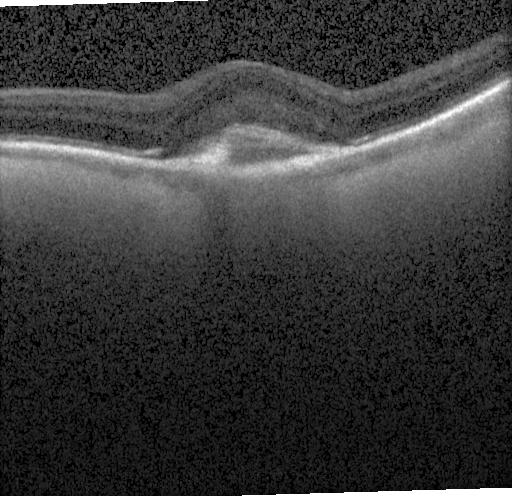 SD-OCT, horizontal scan through the fovea, retinal OCT B-scan, Heidelberg Spectralis OCT system — The scan shows a choroidal neovascular membrane.